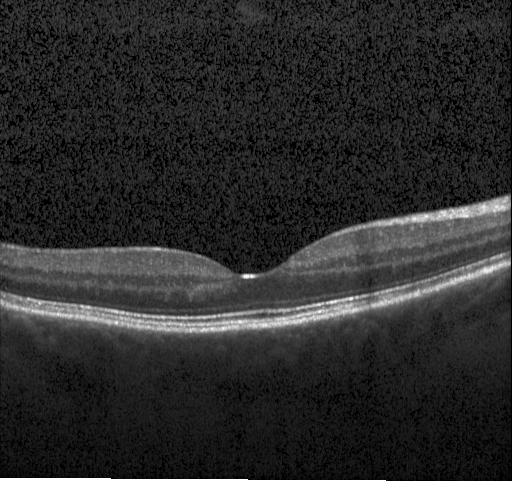

Macular OCT demonstrating no choroidal neovascularization, diabetic macular edema, or drusen.